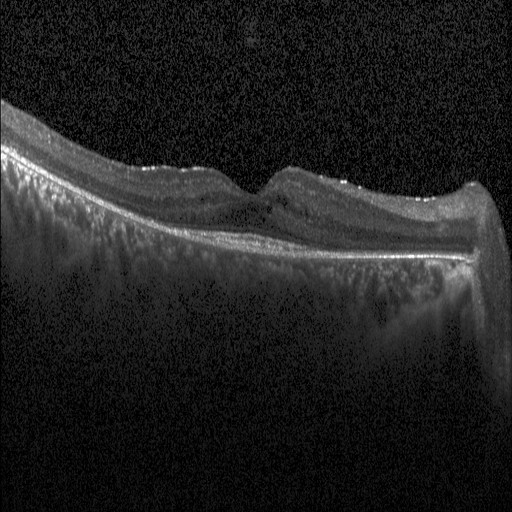

Instrument: Heidelberg Spectralis, SD-OCT, retinal OCT B-scan. Assessment: diabetic macular edema (DME).